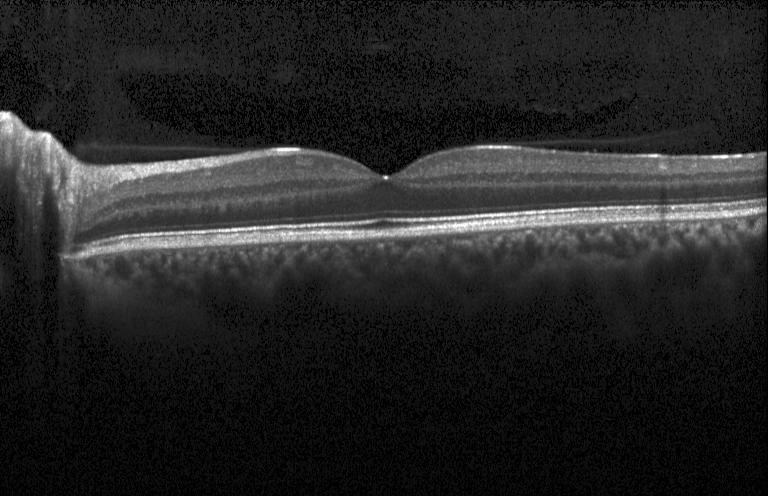
Macular OCT: no choroidal neovascularization, no diabetic macular edema, and no drusen.